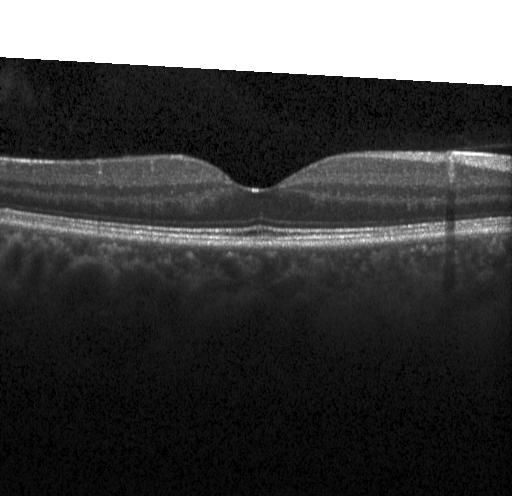

Macular OCT: neither choroidal neovascularization, diabetic macular edema, nor drusen.